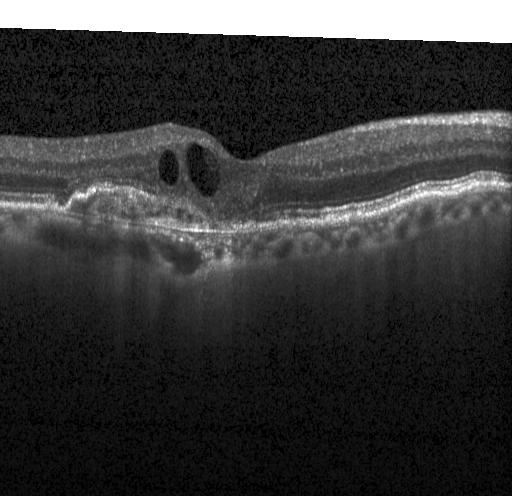

Macular scan. OCT line scan. Instrument: Heidelberg Spectralis. SD-OCT. OCT finding: a choroidal neovascular membrane.